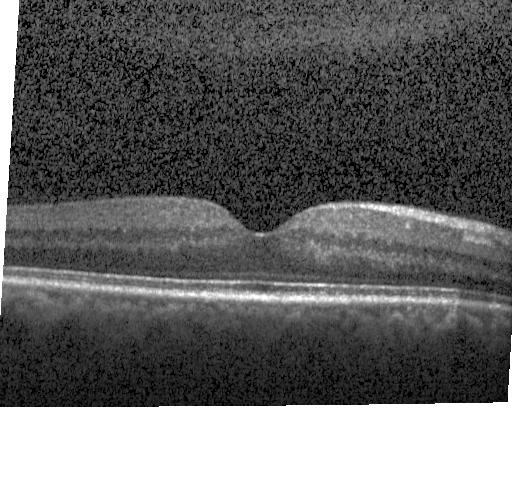

OCT B-scan; spectral-domain optical coherence tomography; through the macula; instrument: Heidelberg Spectralis — Diagnosis: no CNV, DME, or drusen.